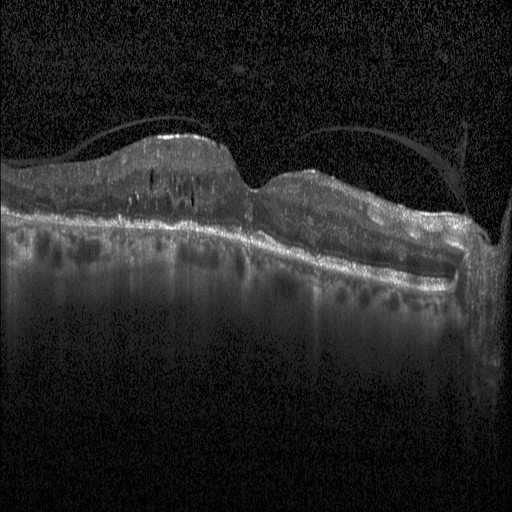
Heidelberg Spectralis OCT system, OCT line scan — Impression: diabetic macular edema.